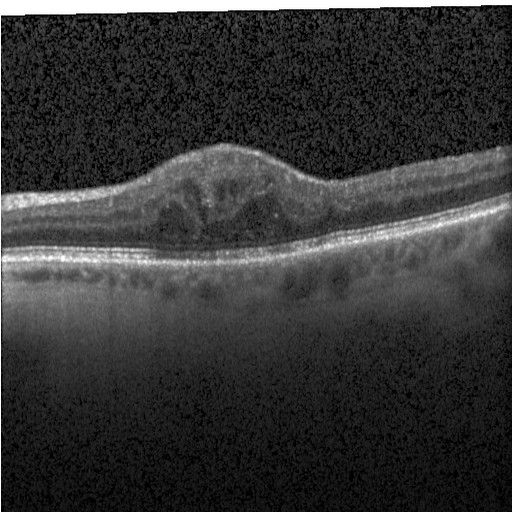
Instrument: Heidelberg Spectralis, retinal OCT B-scan, macular scan, spectral-domain OCT. Assessment: DME.